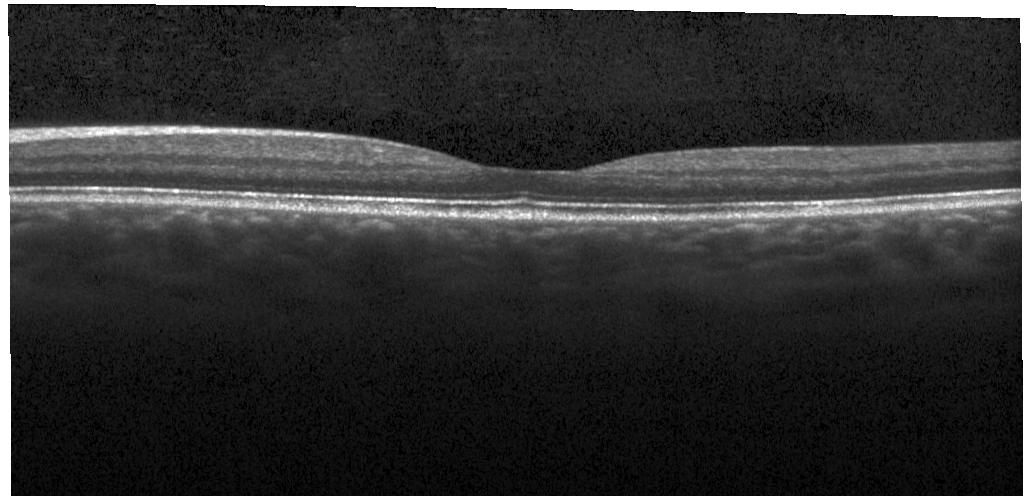
Diagnosis: no evidence of choroidal neovascularization, diabetic macular edema, or drusen.